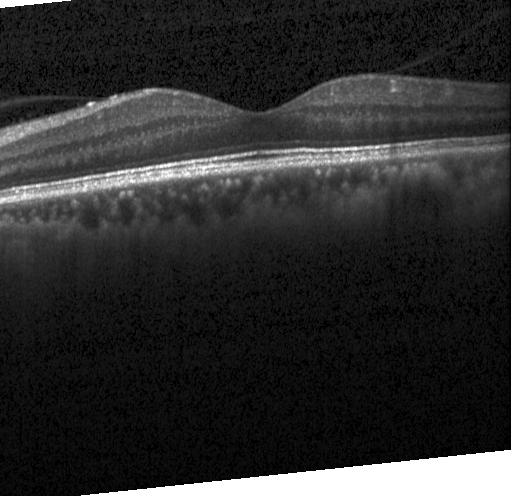

No CNV, DME, or drusen.